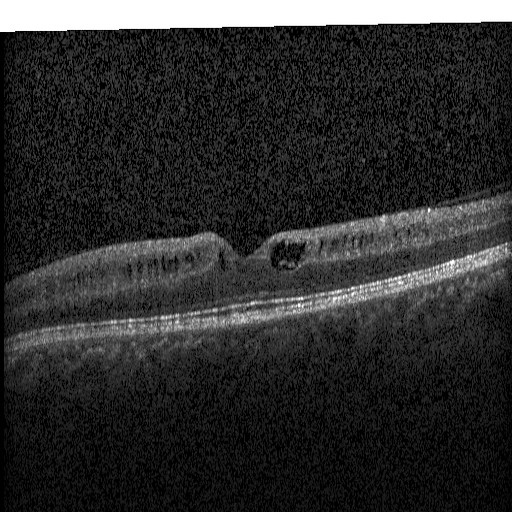

Spectral-domain OCT · retinal OCT cross-section · Heidelberg Spectralis · through the macula — Diabetic macular edema.